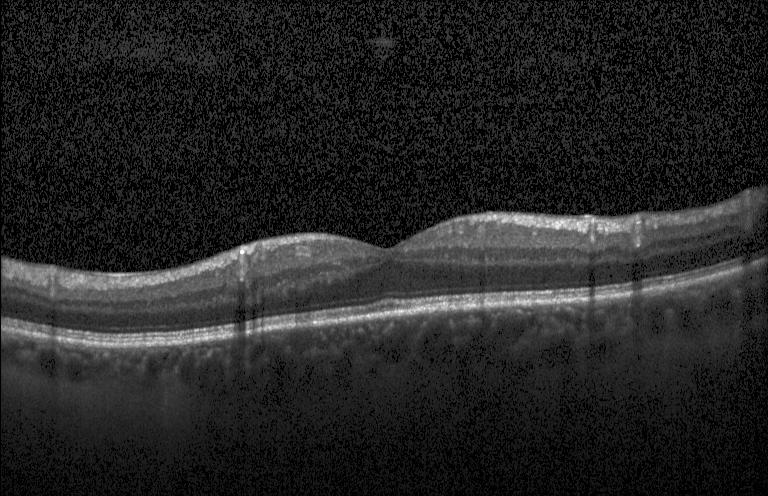
Impression: no choroidal neovascularization, no diabetic macular edema, and no drusen.